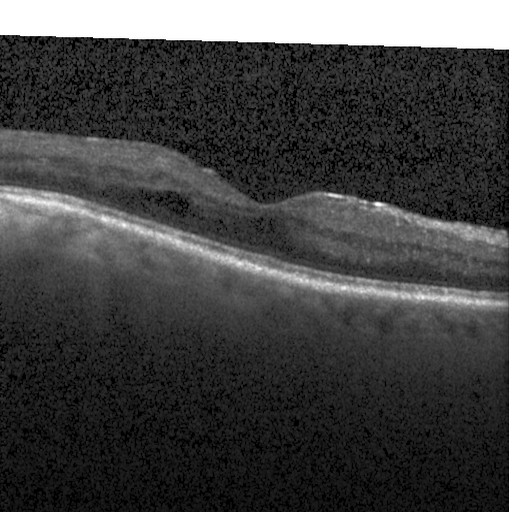 Spectral-domain OCT, retinal OCT B-scan.
Macular OCT: diabetic macular edema (DME).